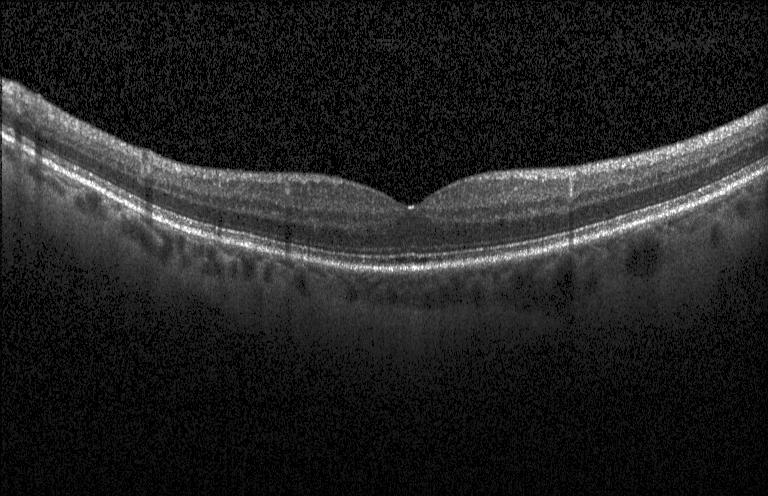

OCT line scan · instrument: Heidelberg Spectralis — This B-scan demonstrates no evidence of CNV, DME, or drusen.